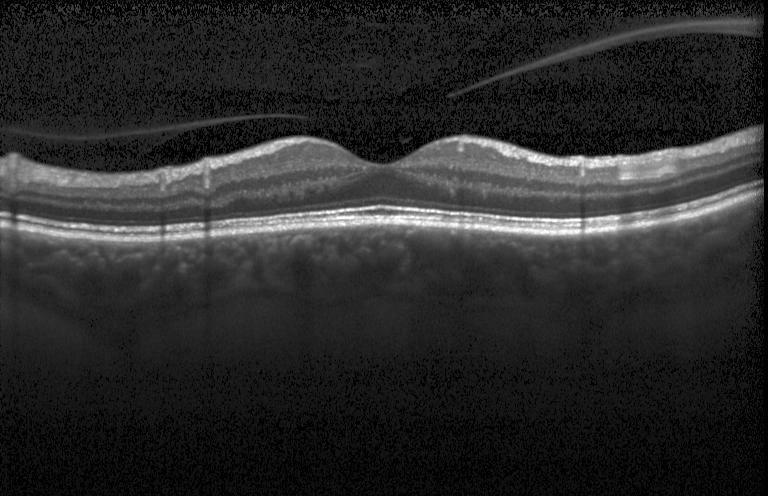

Optical coherence tomography scan; spectral-domain optical coherence tomography; through the macula; instrument: Heidelberg Spectralis
Finding: no CNV, no DME, and no drusen.